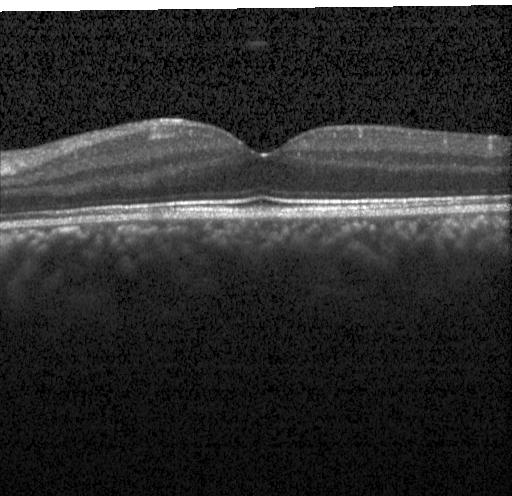

OCT B-scan showing no evidence of CNV, DME, or drusen.